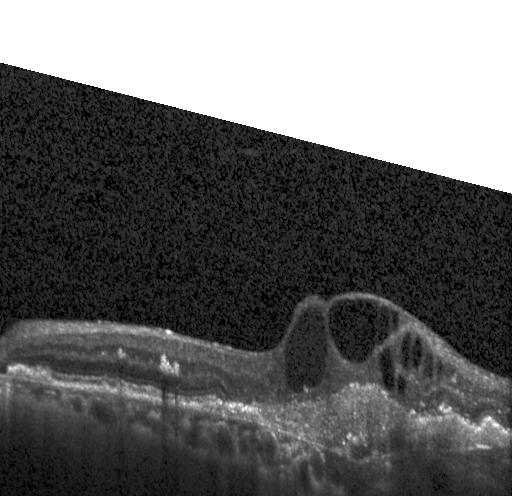
Choroidal neovascularization (CNV).